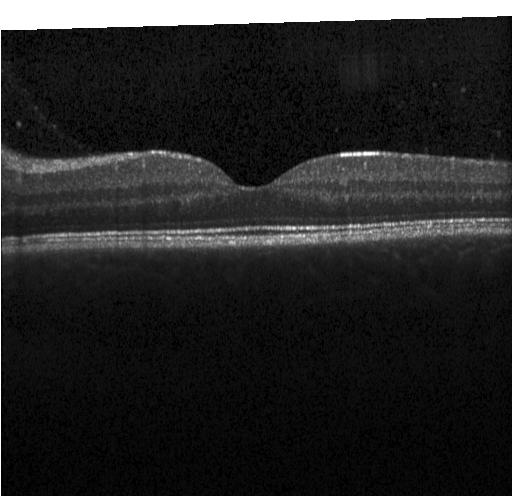 Optical coherence tomography scan. Diagnosis: no choroidal neovascularization, no diabetic macular edema, and no drusen.